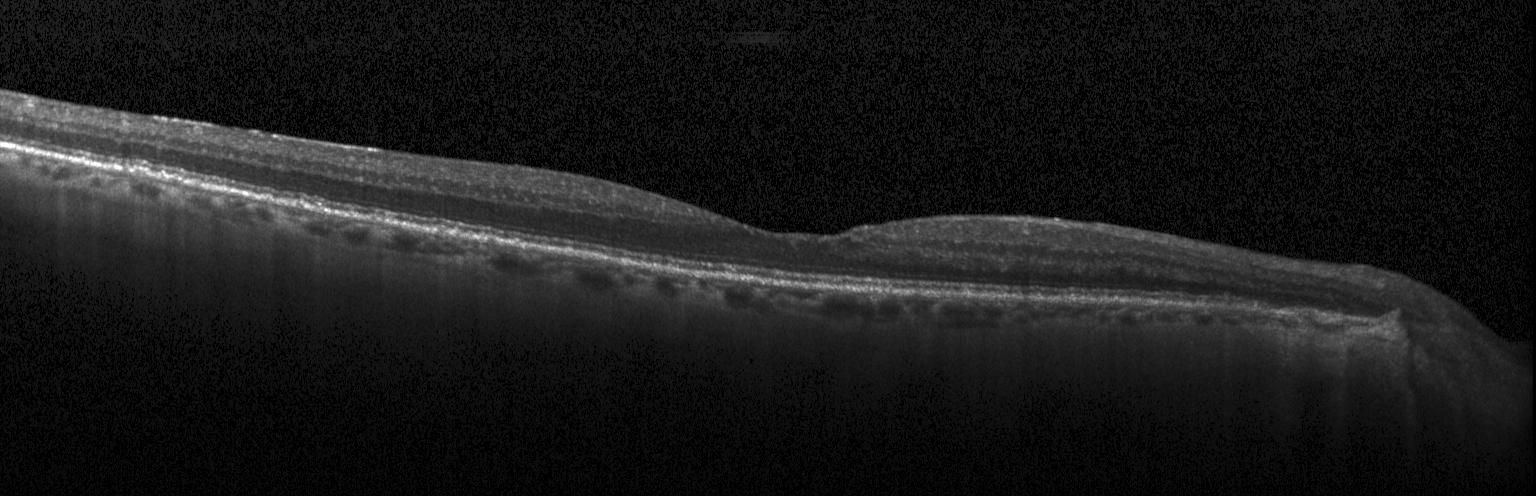 No CNV, no DME, and no drusen.